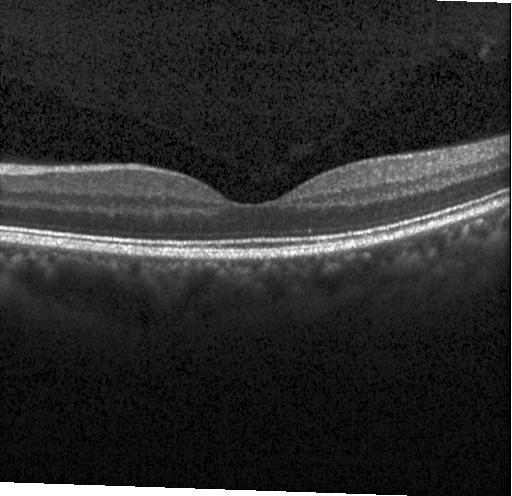 OCT B-scan showing no choroidal neovascularization, no diabetic macular edema, and no drusen.